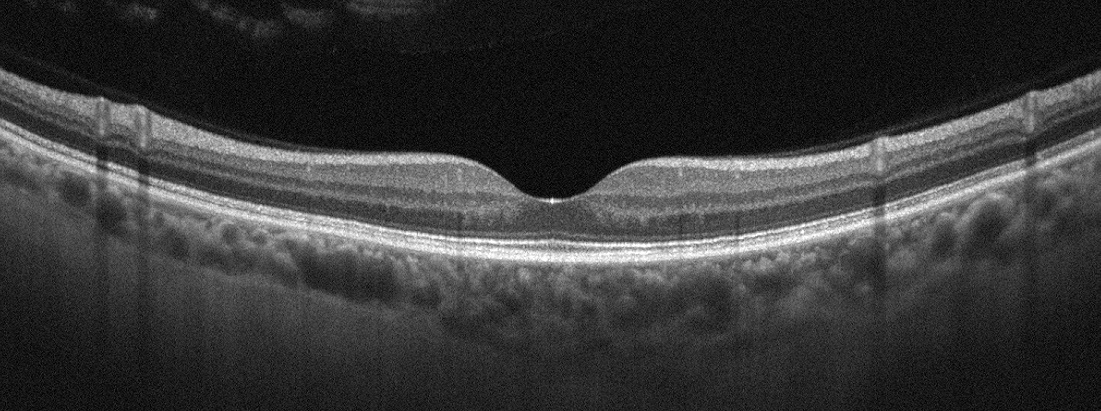 Spectral-domain OCT B-scan: no AMD, DME, ERM, RAO, RVO, or VID.